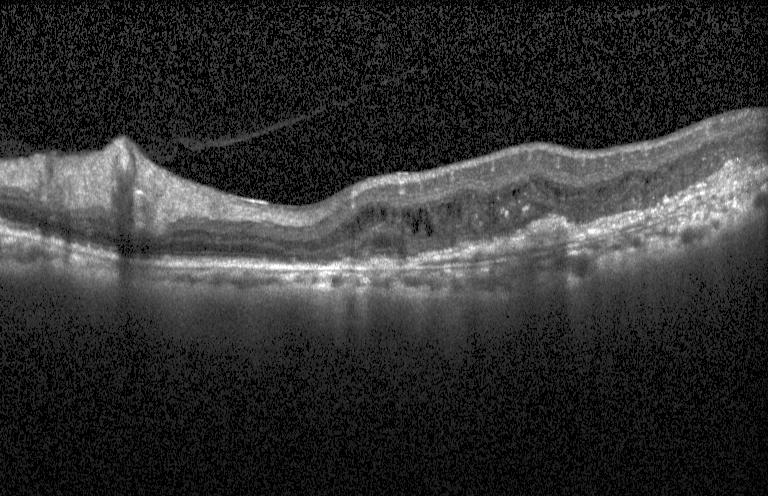

Finding: a choroidal neovascular membrane.